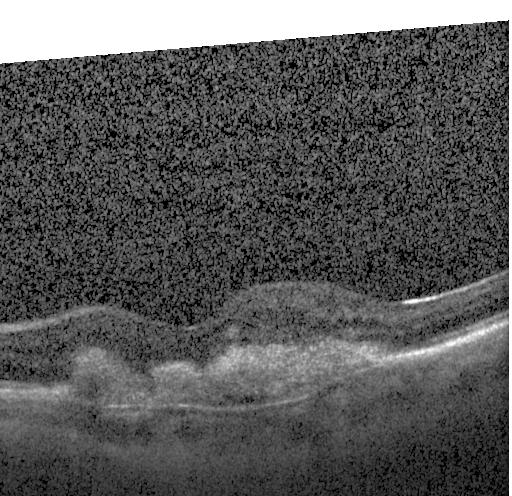
Optical coherence tomography B-scan · spectral-domain OCT. Finding: CNV.